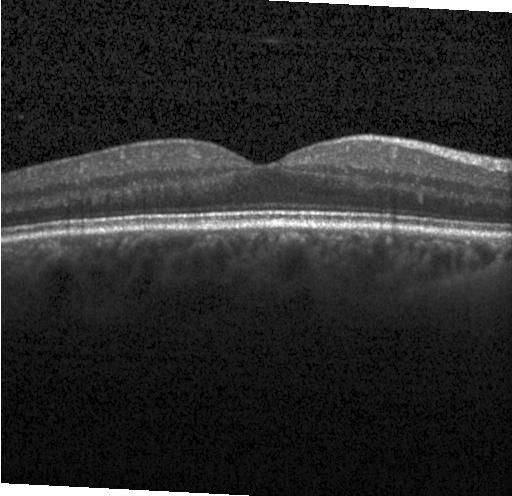

OCT finding: no evidence of choroidal neovascularization, diabetic macular edema, or drusen.